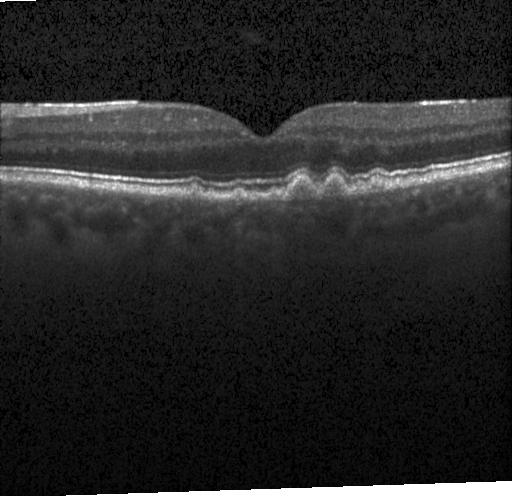

OCT finding: multiple drusen.